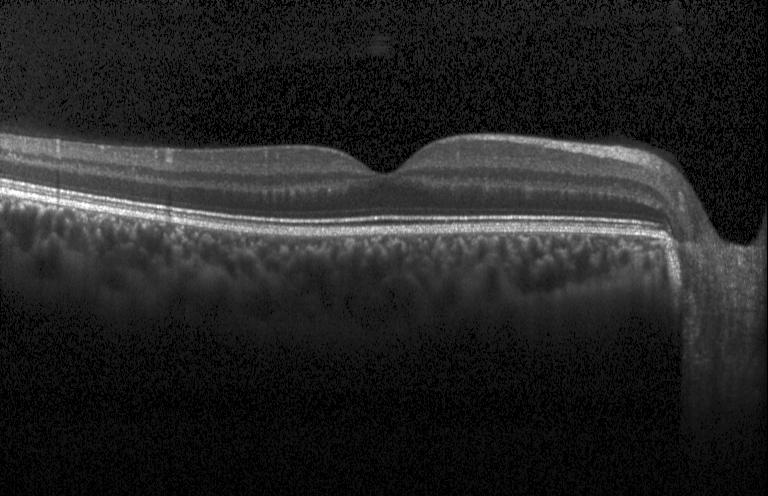

OCT B-scan; centered on the fovea — Assessment: no CNV, DME, or drusen.